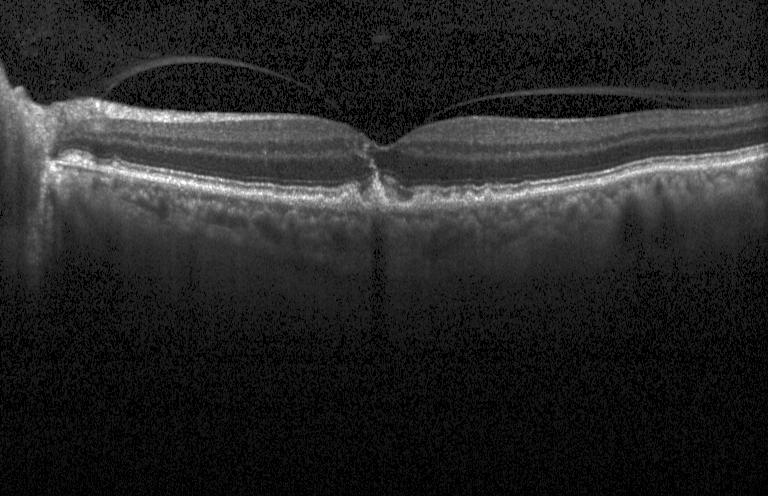 Spectral-domain OCT B-scan: drusen.